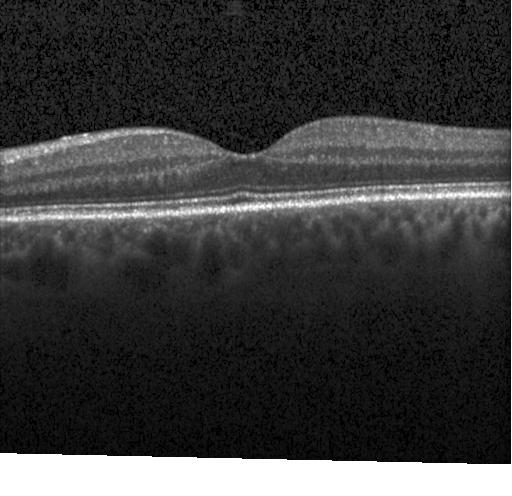

Retinal OCT cross-section — Dx: no CNV, no DME, and no drusen.